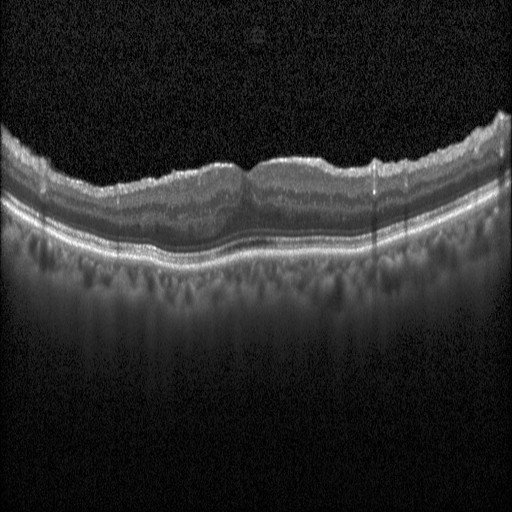 The scan shows DME.